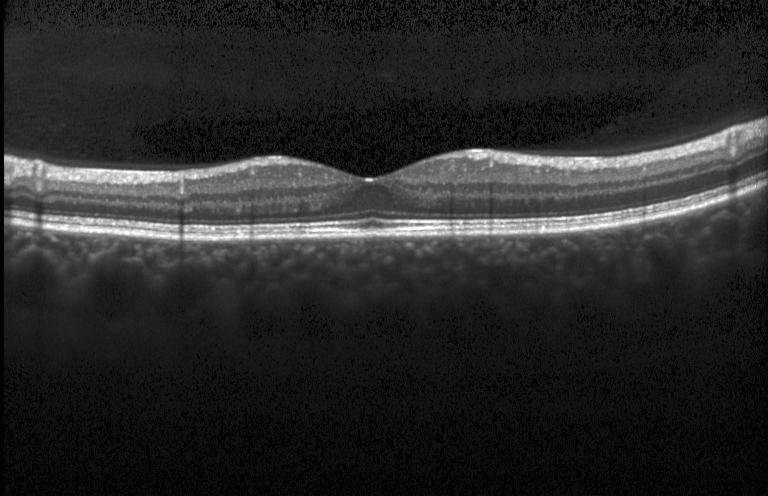
OCT B-scan
Dx: no CNV, DME, or drusen.